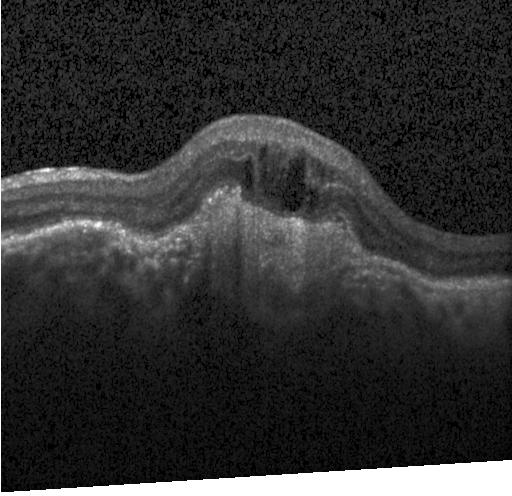

OCT scan showing choroidal neovascularization.